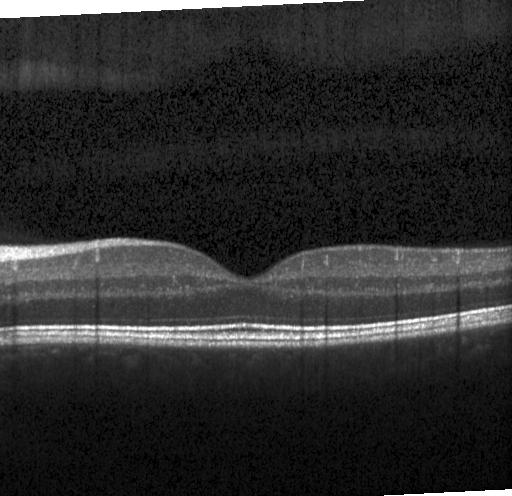

Retinal OCT B-scan. Finding: no CNV, DME, or drusen.